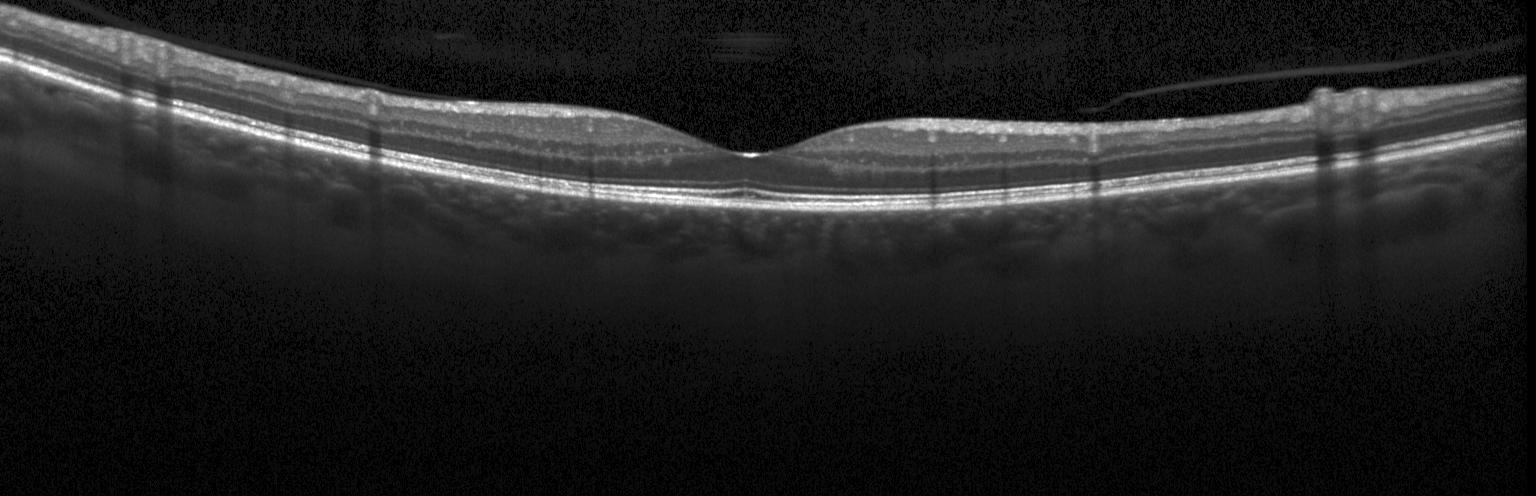

Acquired on a Heidelberg Spectralis; spectral-domain optical coherence tomography; OCT line scan; macular scan — The scan shows no evidence of CNV, DME, or drusen.